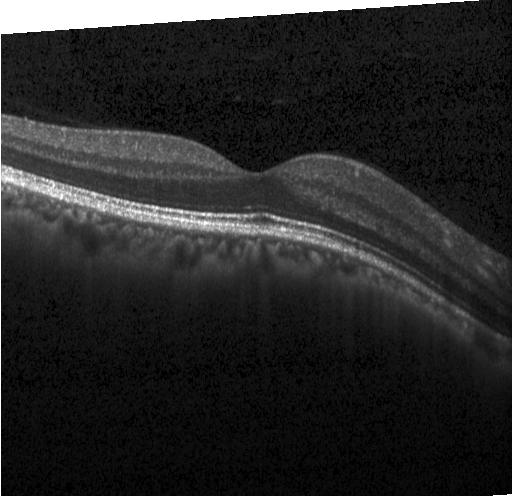

Retinal OCT cross-section showing no choroidal neovascularization, no diabetic macular edema, and no drusen.